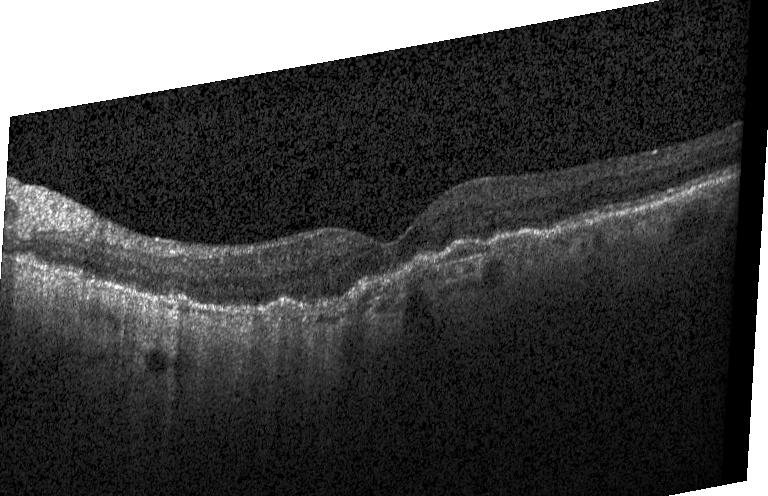
Optical coherence tomography B-scan
Diagnosis: CNV.